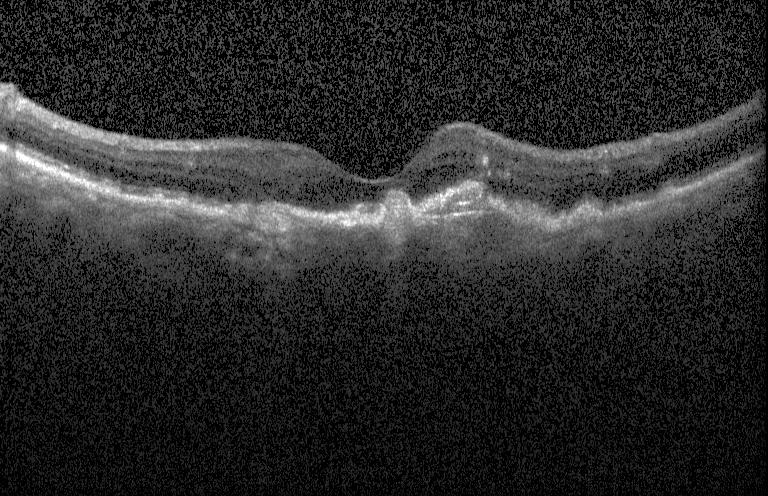
Through the macula. Retinal OCT B-scan. Heidelberg Spectralis. SD-OCT.
This B-scan demonstrates a choroidal neovascular membrane.